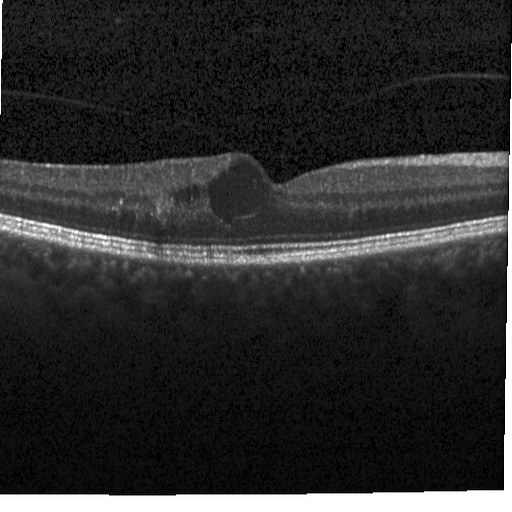
Finding: diabetic macular edema (DME).